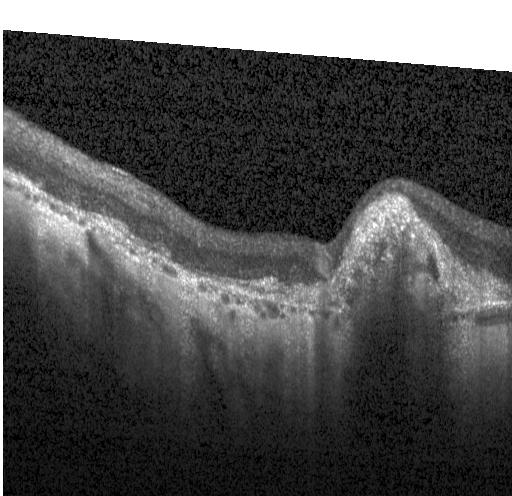

Impression: choroidal neovascularization.